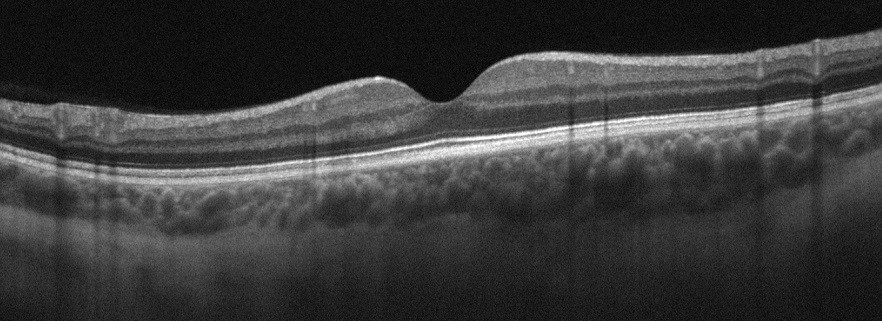 Impression: no AMD, DME, ERM, RAO, RVO, or VID.